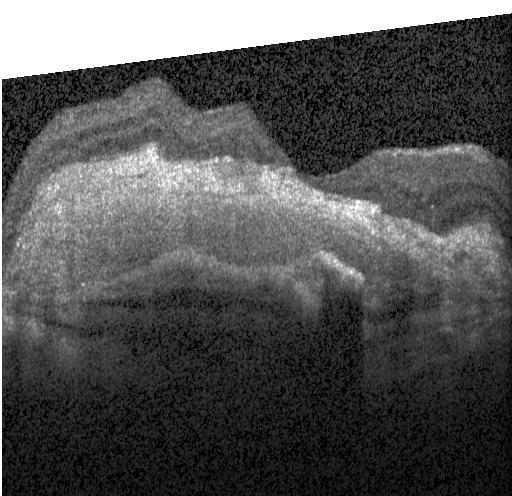

Retinal OCT B-scan — Impression: CNV.